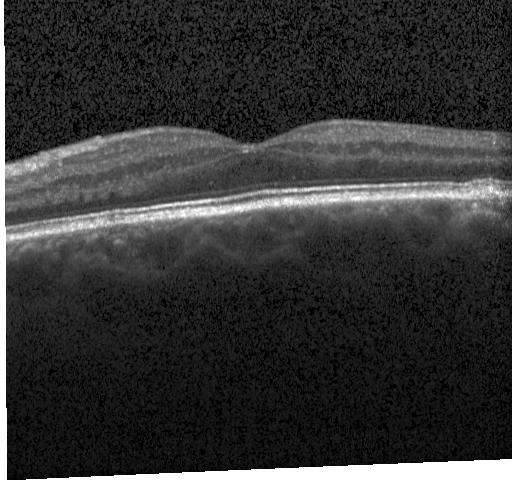 Impression: neither CNV, DME, nor drusen.